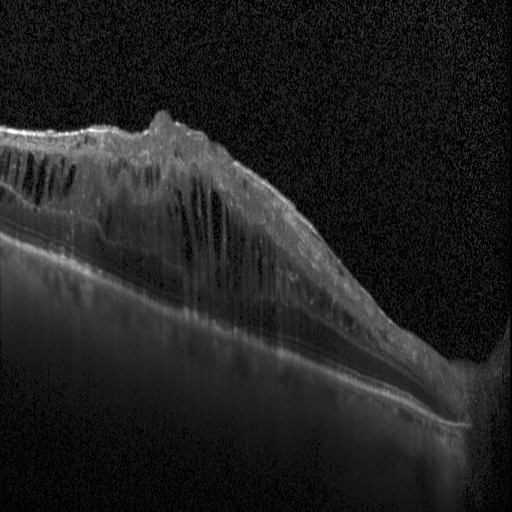

SD-OCT, Heidelberg Spectralis, optical coherence tomography B-scan, horizontal scan through the fovea
Impression: diabetic macular edema.